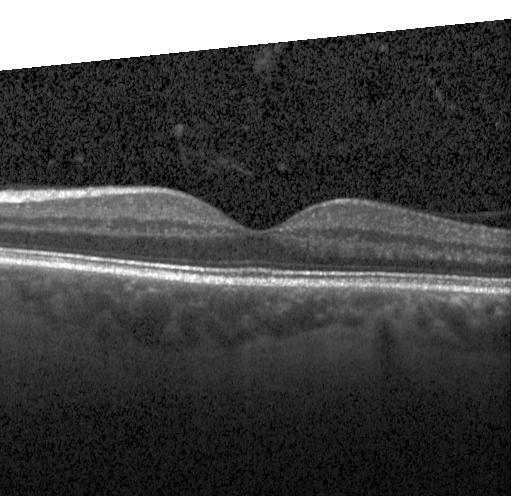

SD-OCT. Optical coherence tomography B-scan
OCT finding: no choroidal neovascularization, diabetic macular edema, or drusen.